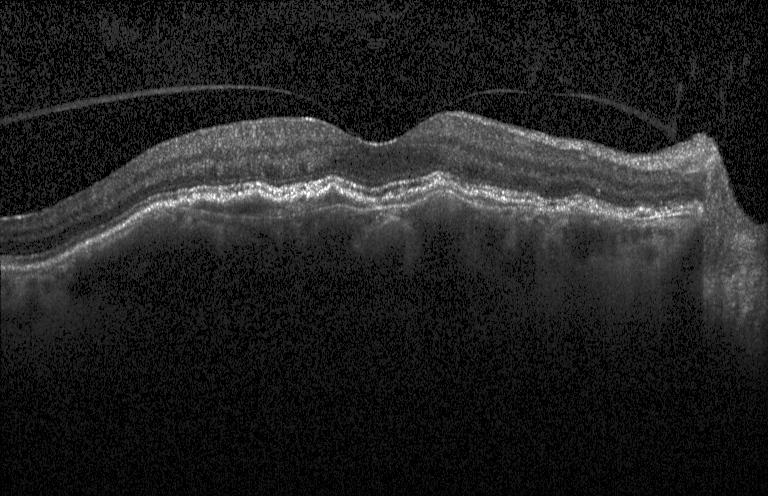
Centered on the fovea · retinal OCT B-scan · spectral-domain OCT · acquired on a Heidelberg Spectralis
Dx: a choroidal neovascular membrane.